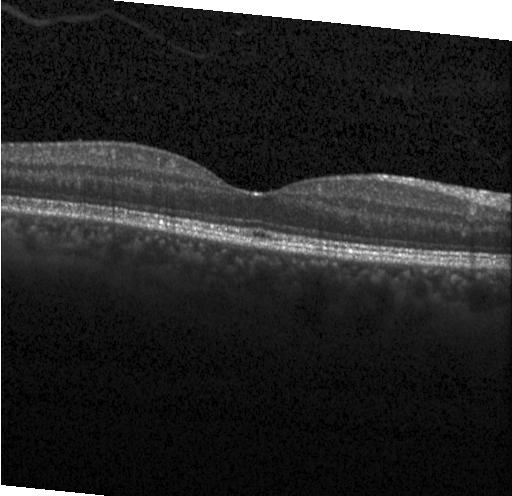
Optical coherence tomography scan; acquired on a Heidelberg Spectralis; through the macula — OCT finding: no evidence of CNV, DME, or drusen.